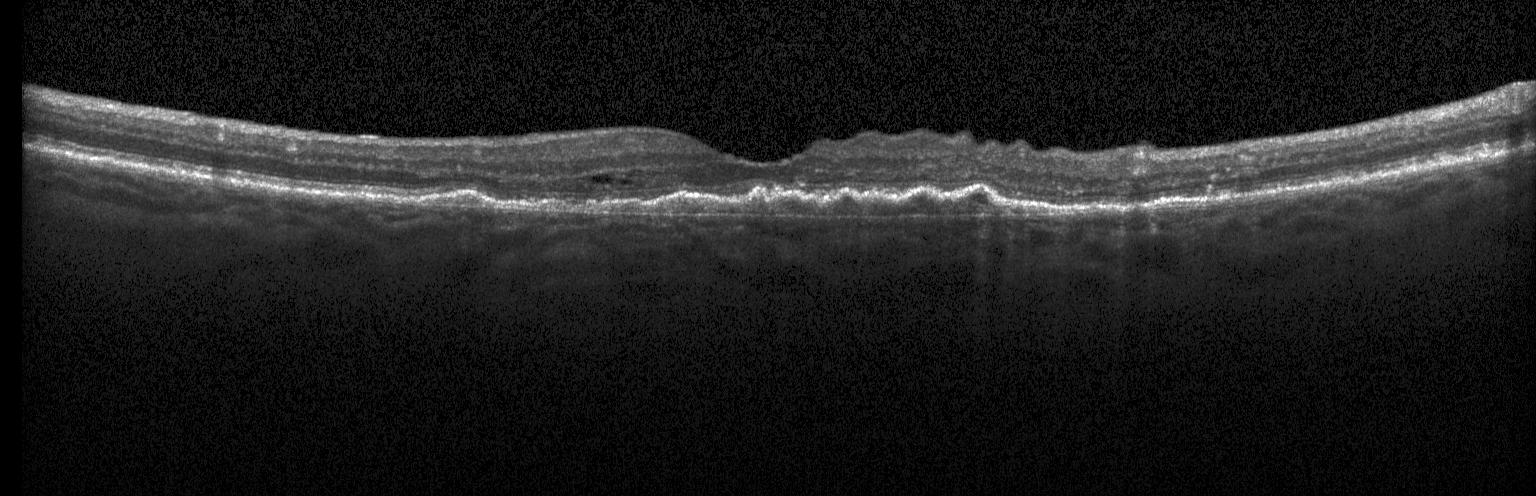
OCT line scan; Heidelberg Spectralis; through the macula. This B-scan demonstrates a choroidal neovascular membrane.